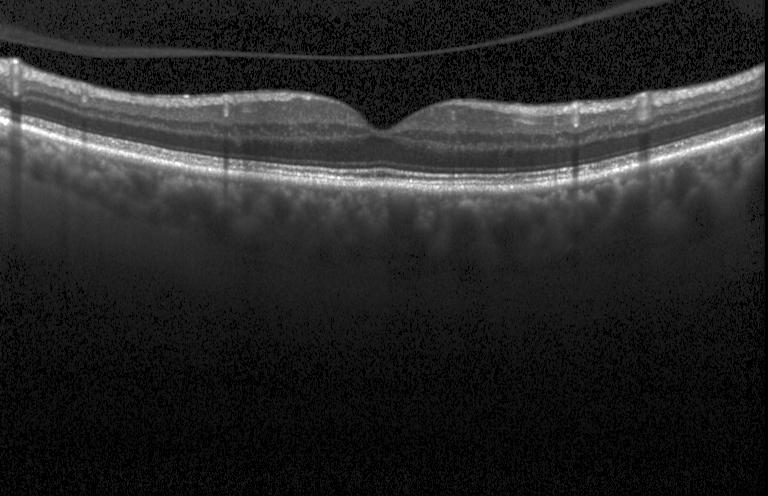

Acquired on a Heidelberg Spectralis, centered on the fovea, retinal OCT cross-section, spectral-domain OCT.
Impression: no choroidal neovascularization, no diabetic macular edema, and no drusen.